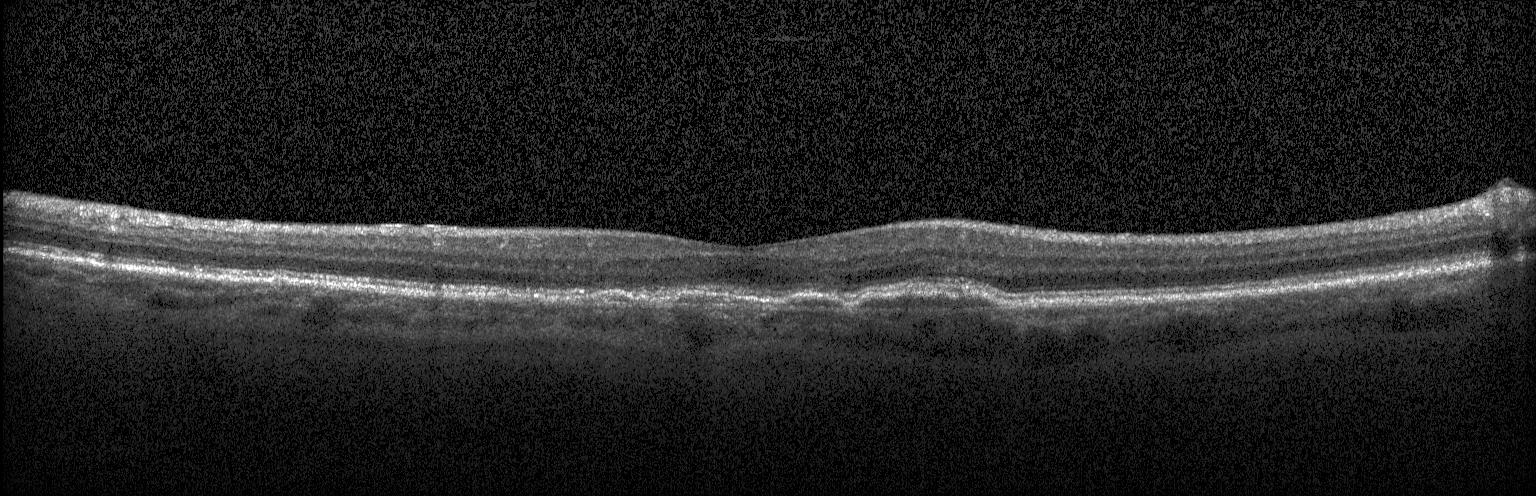

CNV.